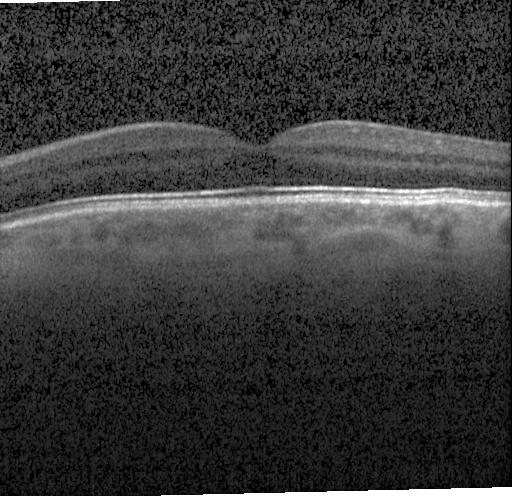 The scan shows neither CNV, DME, nor drusen.